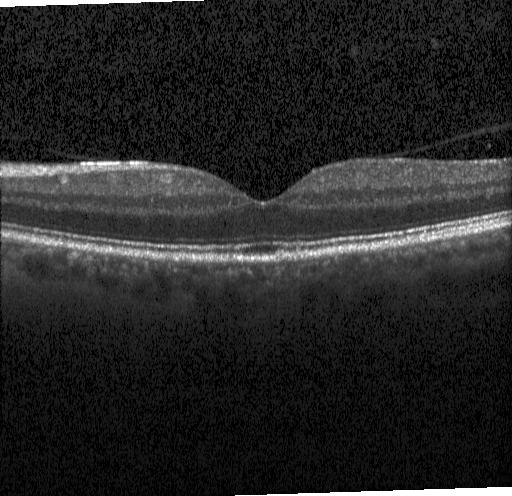 Macular OCT: no evidence of choroidal neovascularization, diabetic macular edema, or drusen.